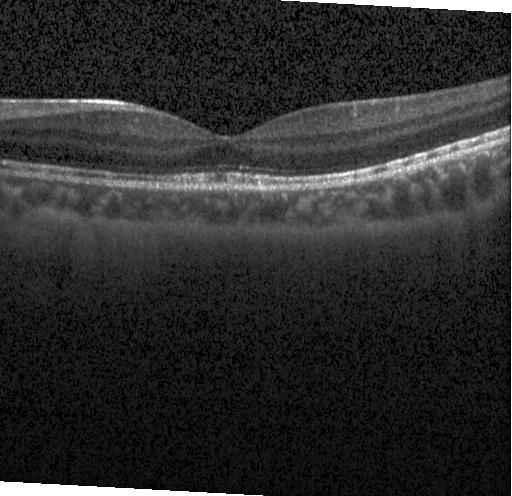

Retinal OCT cross-section · horizontal scan through the fovea
No evidence of choroidal neovascularization, diabetic macular edema, or drusen.